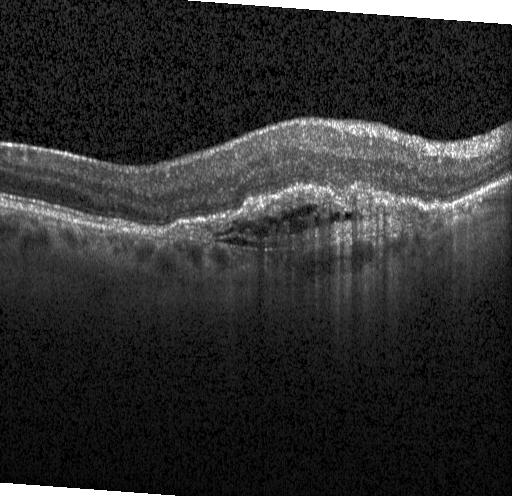 Diagnosis: CNV.